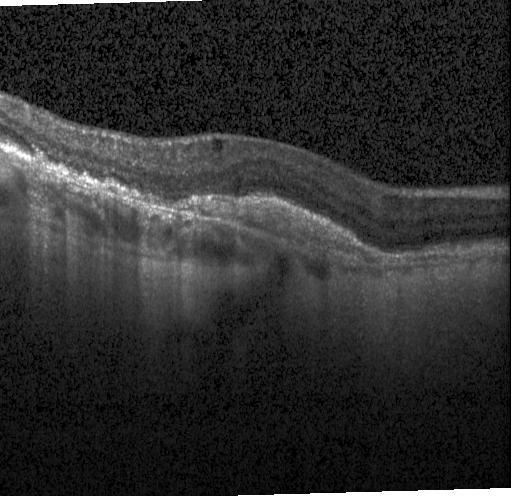 Retinal OCT cross-section showing choroidal neovascularization (CNV).